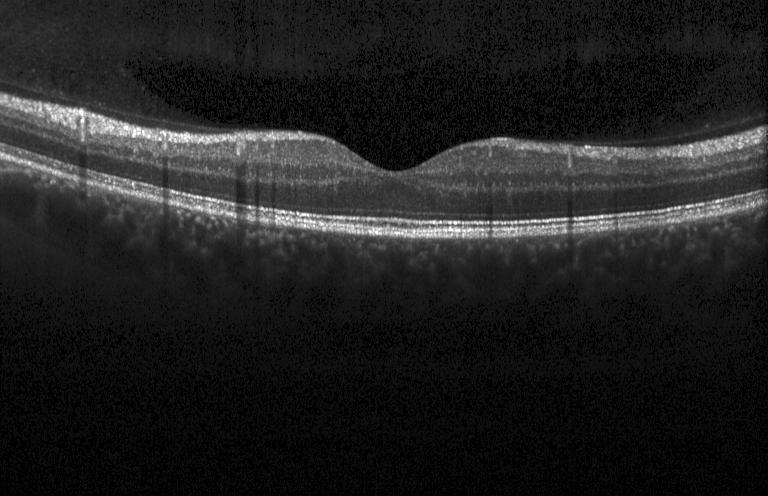
Macular OCT: no choroidal neovascularization, diabetic macular edema, or drusen.